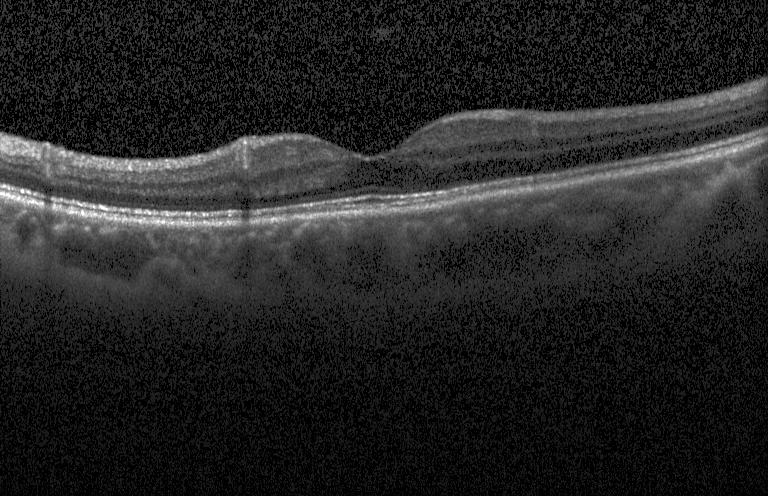 No CNV, no DME, and no drusen.